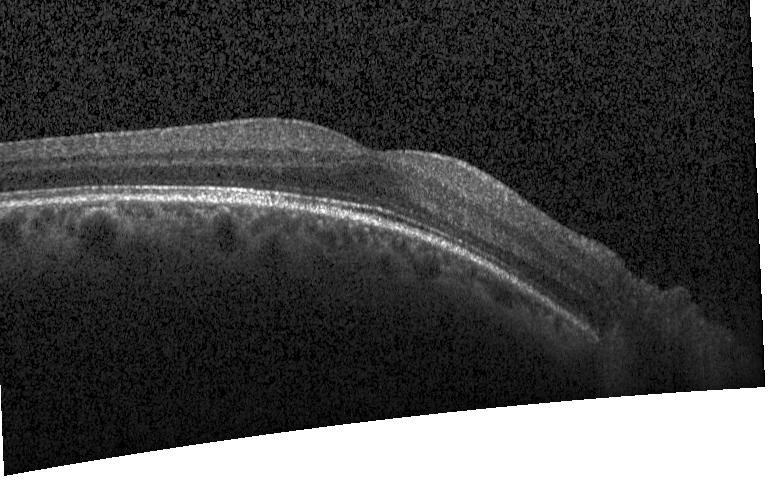

Macular scan. Spectral-domain optical coherence tomography. OCT B-scan. Diagnosis: no choroidal neovascularization, no diabetic macular edema, and no drusen.